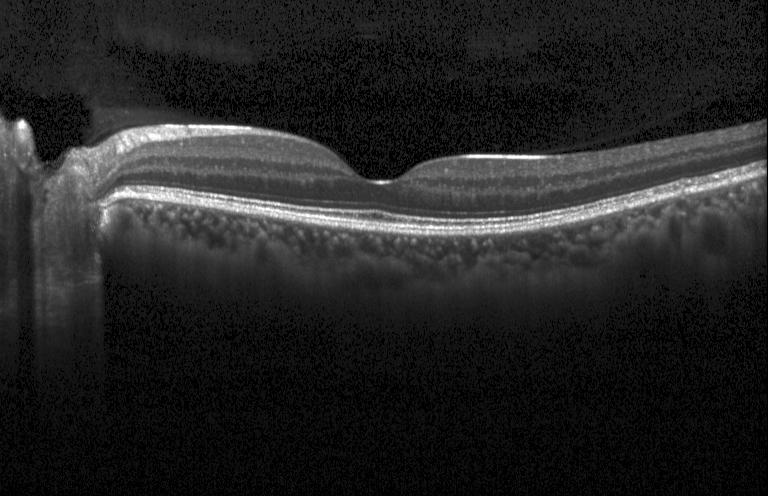
Retinal OCT cross-section · macular scan · spectral-domain optical coherence tomography · Heidelberg Spectralis OCT system.
The scan shows no evidence of choroidal neovascularization, diabetic macular edema, or drusen.